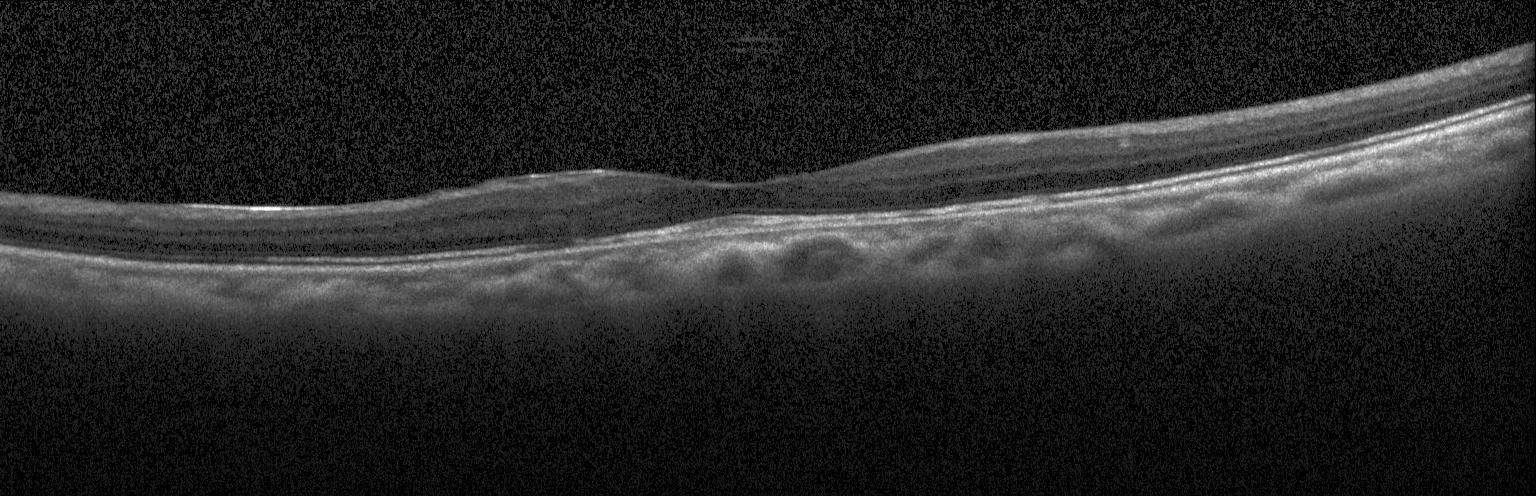

OCT line scan, spectral-domain optical coherence tomography. Impression: no evidence of choroidal neovascularization, diabetic macular edema, or drusen.